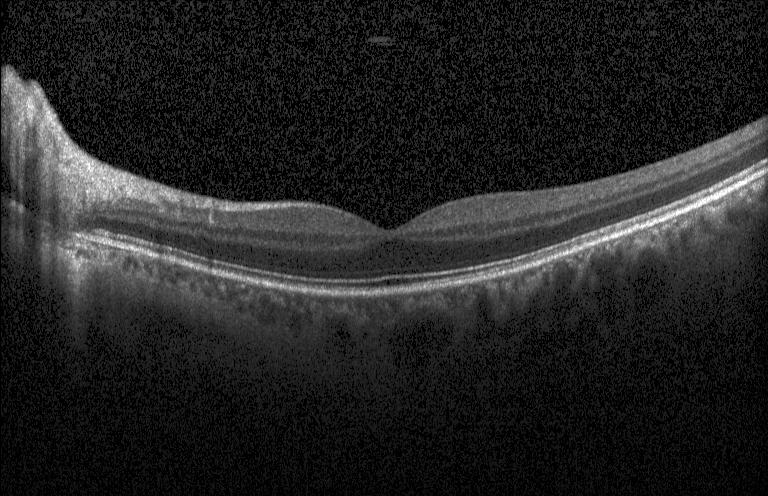
OCT line scan, spectral-domain optical coherence tomography, centered on the fovea. Finding: no evidence of CNV, DME, or drusen.